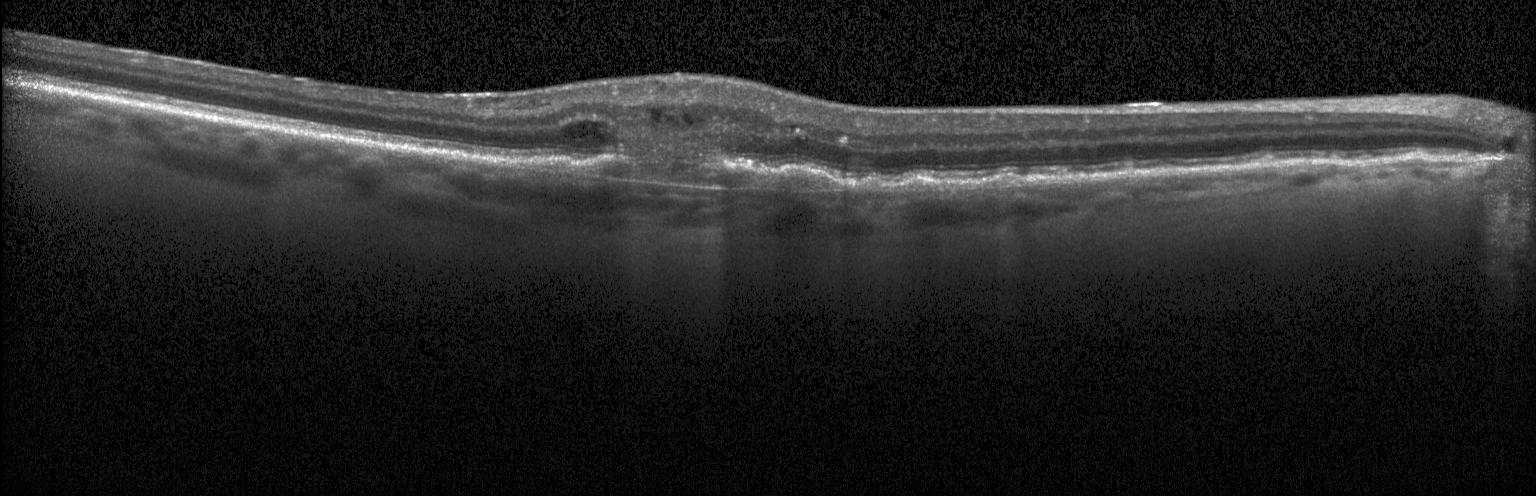 Finding: choroidal neovascularization.